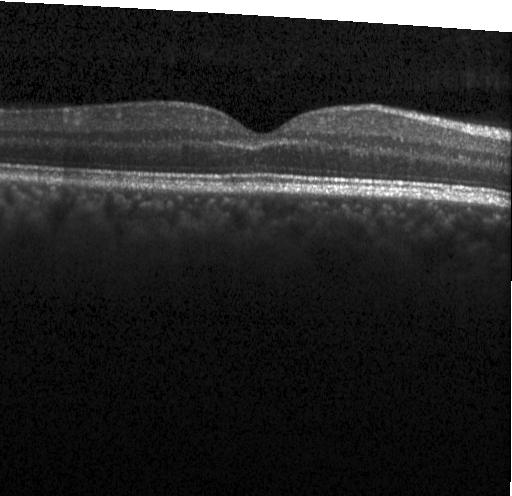

Optical coherence tomography scan. Fovea-centered.
Assessment: neither choroidal neovascularization, diabetic macular edema, nor drusen.